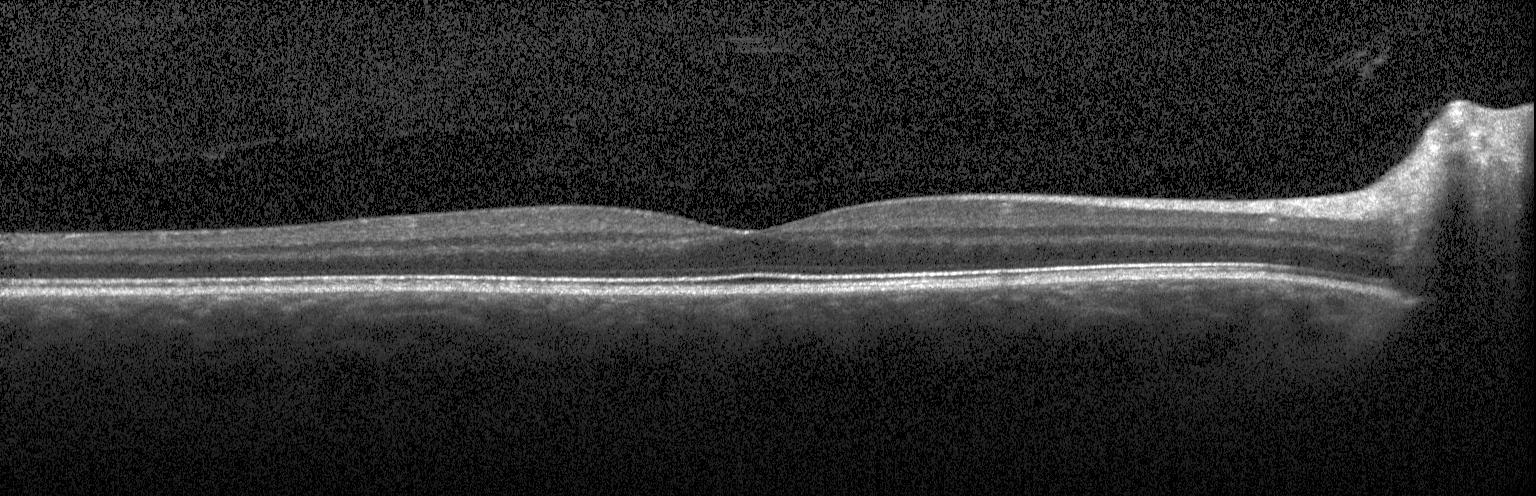
This B-scan demonstrates no CNV, no DME, and no drusen.